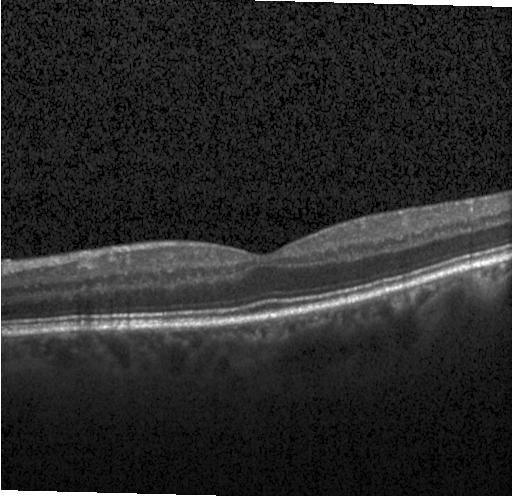
Retinal OCT B-scan. This B-scan demonstrates no CNV, DME, or drusen.